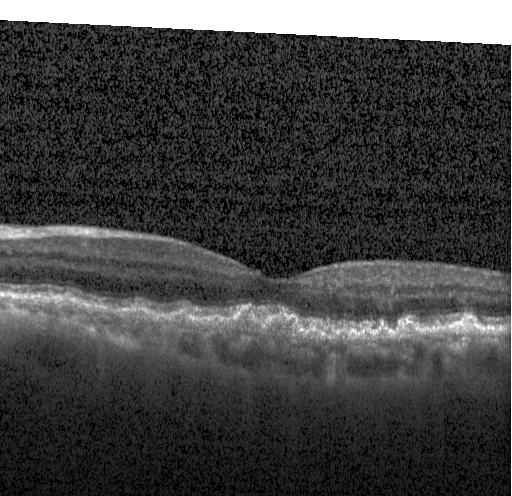

Through the macula, OCT line scan. This B-scan demonstrates sub-RPE drusenoid deposits.